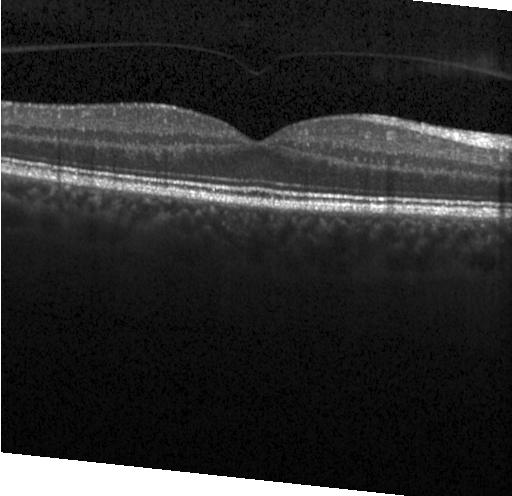
OCT line scan.
Assessment: no choroidal neovascularization, diabetic macular edema, or drusen.